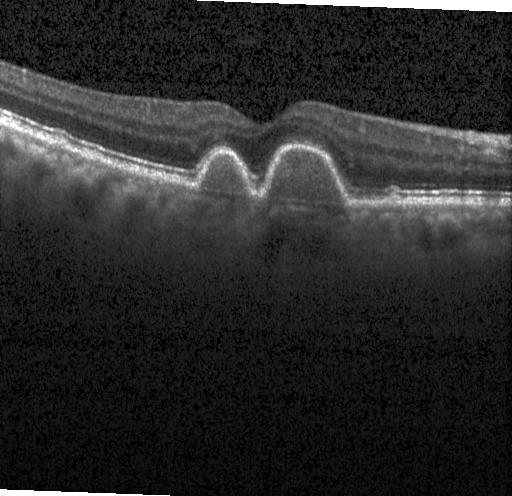

Optical coherence tomography scan.
Assessment: multiple drusen.